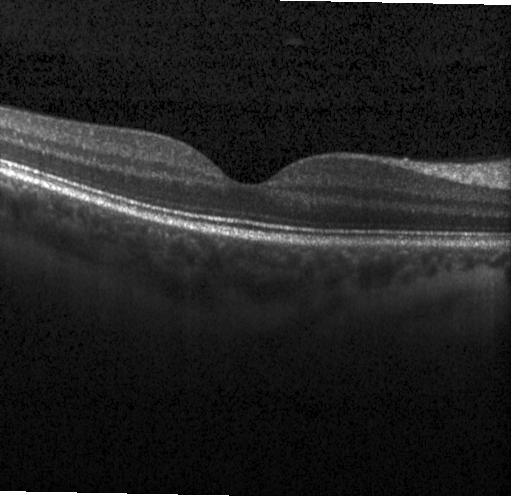
Instrument: Heidelberg Spectralis · SD-OCT · optical coherence tomography B-scan · centered on the fovea. Finding: no evidence of choroidal neovascularization, diabetic macular edema, or drusen.